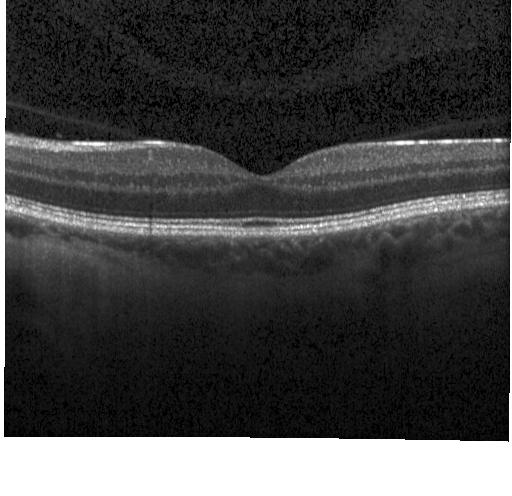

OCT B-scan. No CNV, DME, or drusen.